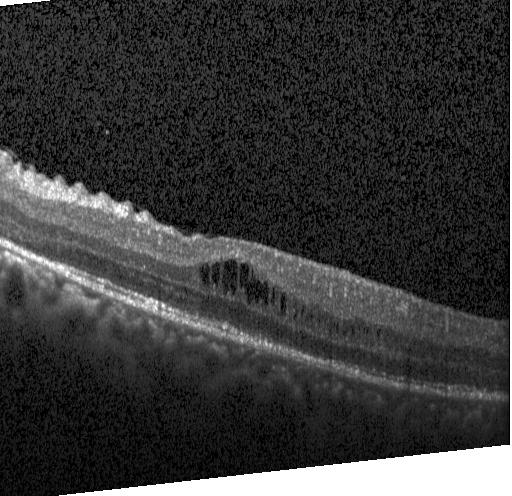
Heidelberg Spectralis; optical coherence tomography scan. The scan shows diabetic macular edema (DME).